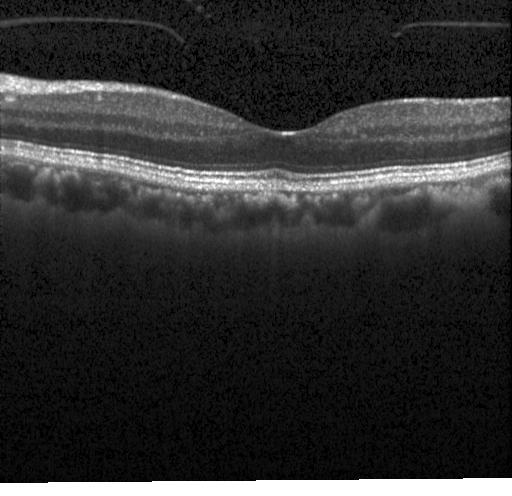

Retinal OCT B-scan — Dx: no evidence of choroidal neovascularization, diabetic macular edema, or drusen.